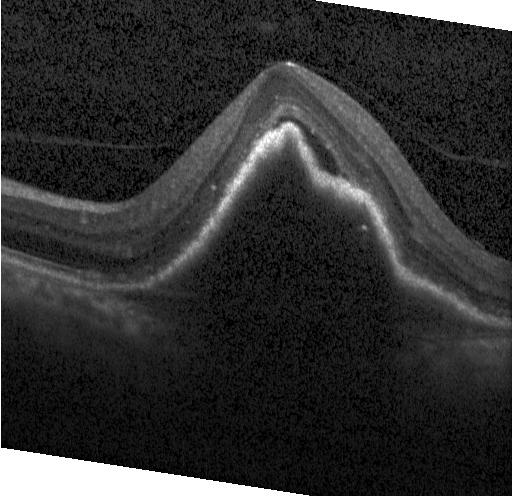 OCT B-scan. Heidelberg Spectralis OCT system. SD-OCT.
OCT finding: a choroidal neovascular membrane.